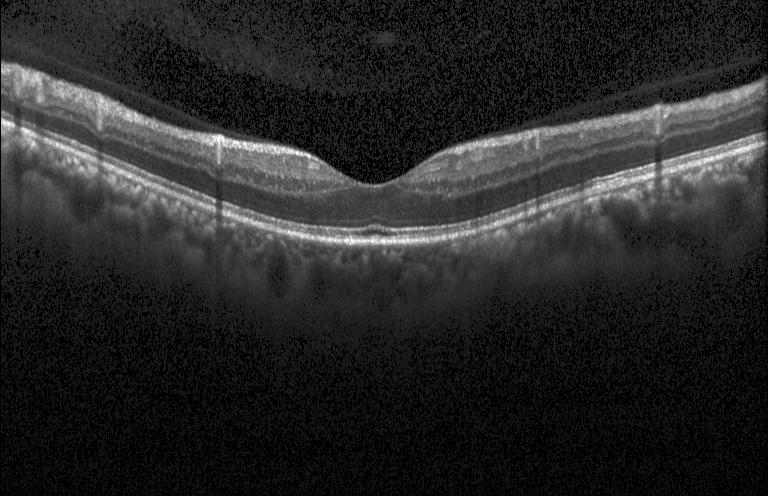 Finding: no choroidal neovascularization, diabetic macular edema, or drusen.